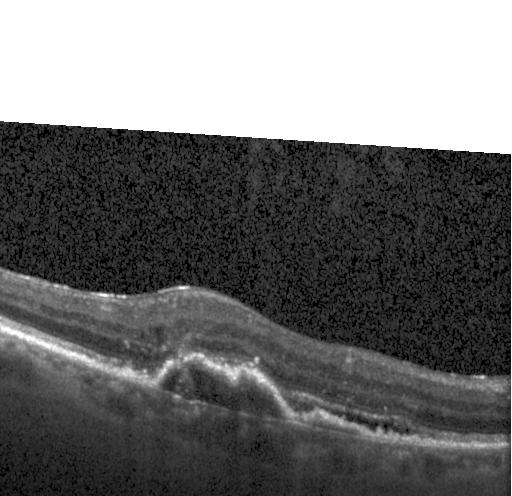 Optical coherence tomography scan — Choroidal neovascularization (CNV).